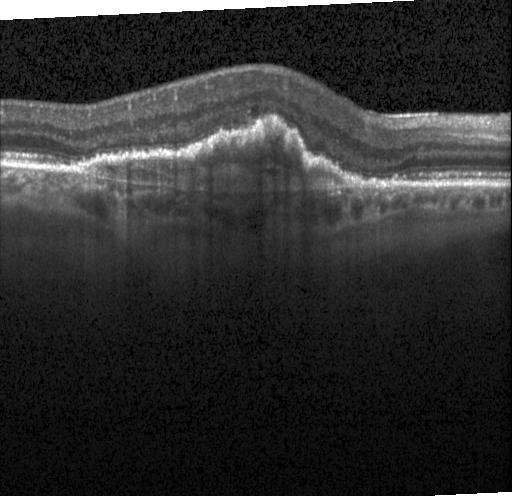 Retinal OCT cross-section showing CNV.